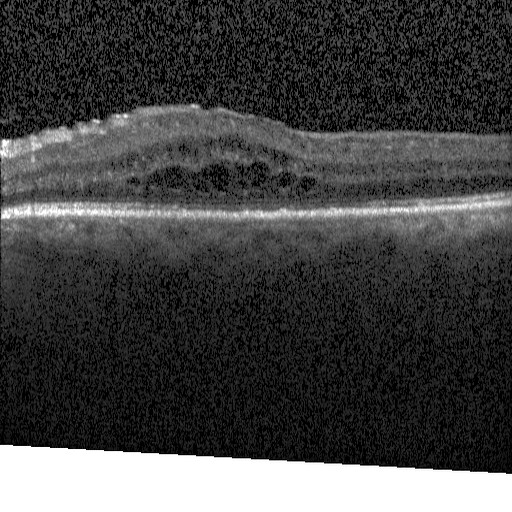
Retinal OCT B-scan, fovea-centered. Diagnosis: diabetic macular edema.